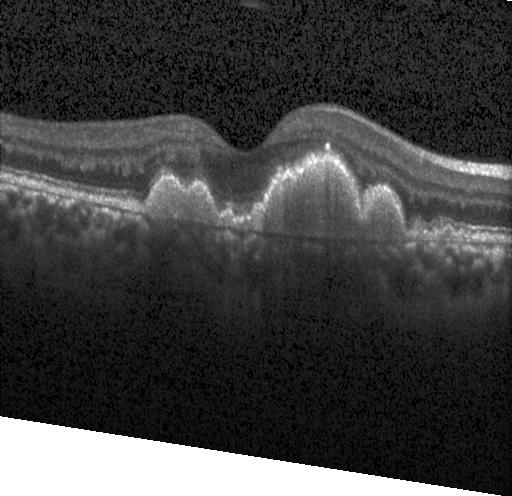
Optical coherence tomography scan. Spectral-domain optical coherence tomography. OCT finding: sub-RPE drusenoid deposits.